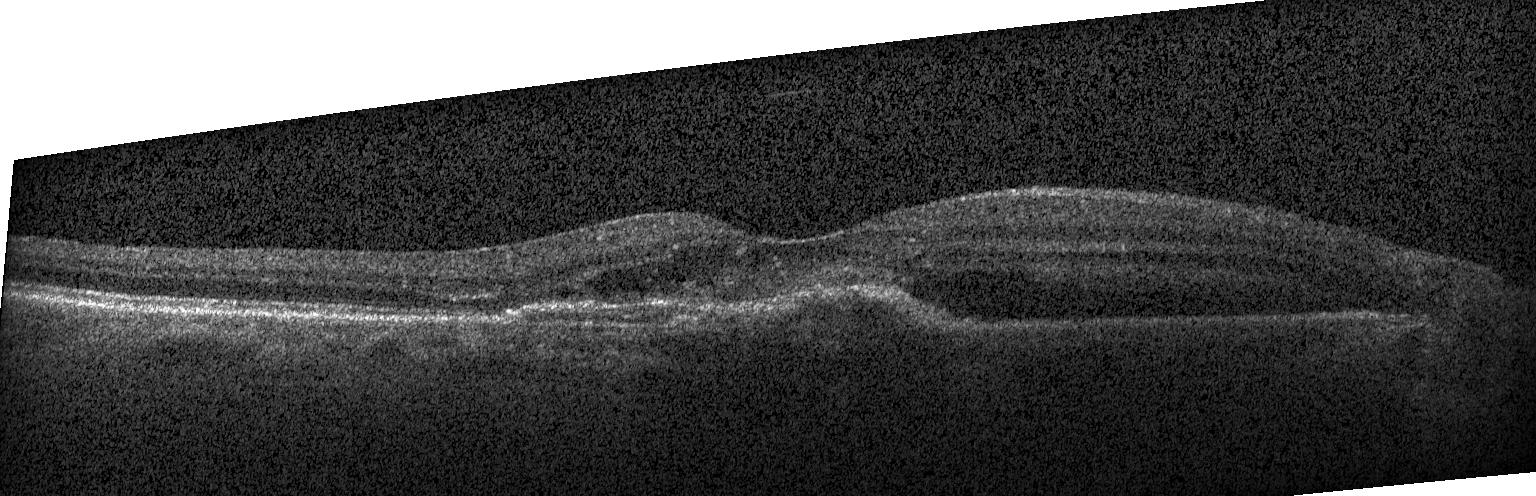
OCT B-scan, SD-OCT.
Finding: a choroidal neovascular membrane.